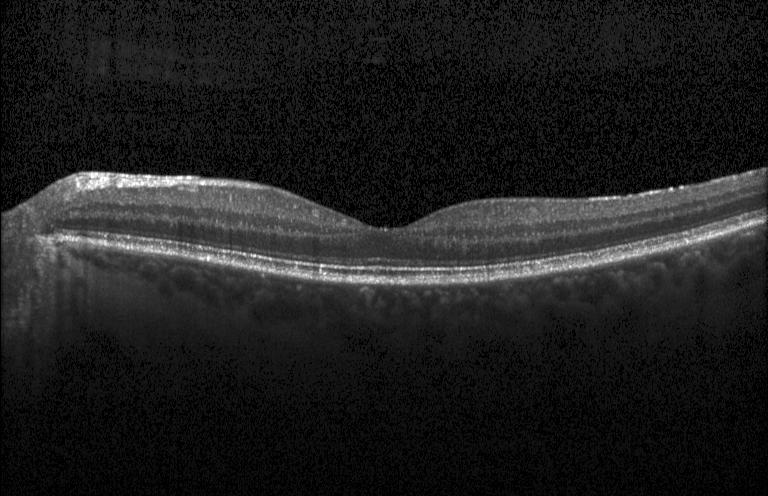
Retinal OCT cross-section showing no choroidal neovascularization, diabetic macular edema, or drusen.